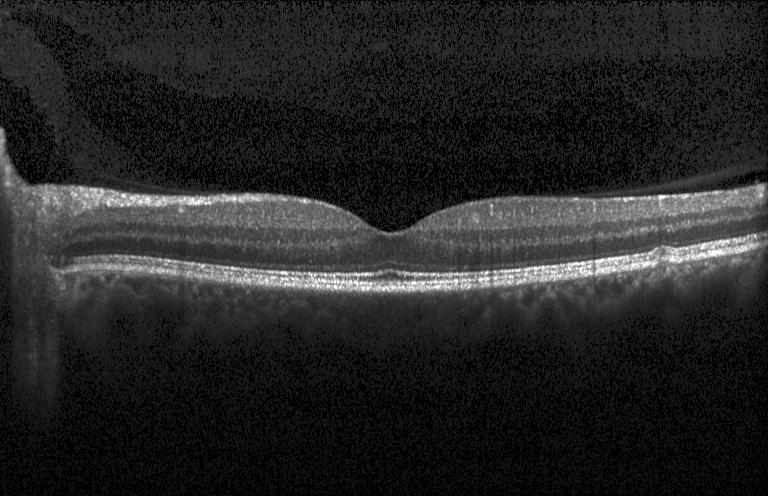

Dx: sub-RPE drusenoid deposits.